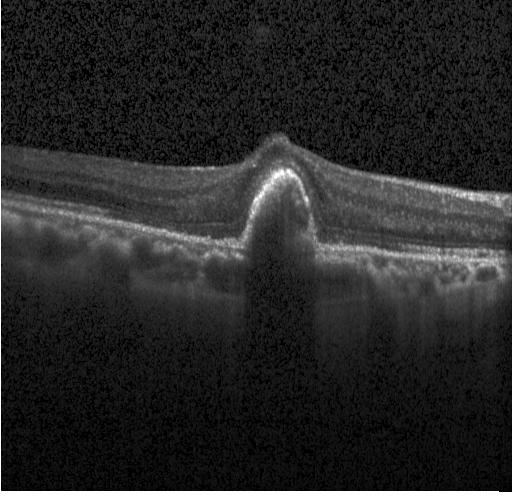
Finding: a choroidal neovascular membrane.